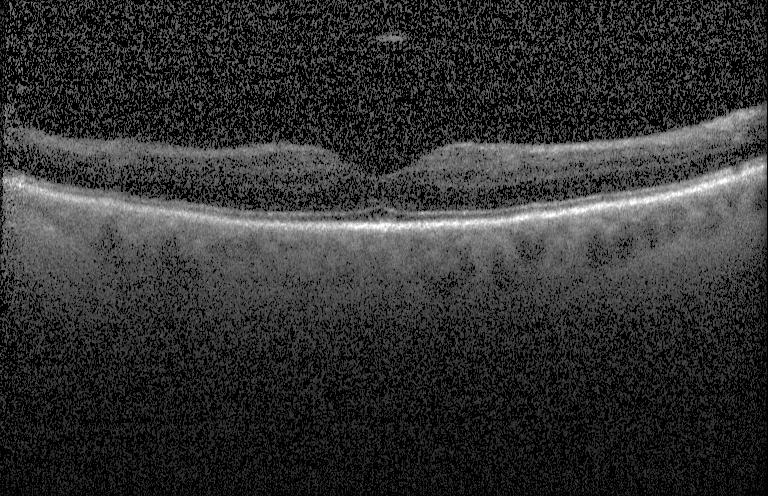 OCT B-scan showing no evidence of choroidal neovascularization, diabetic macular edema, or drusen.